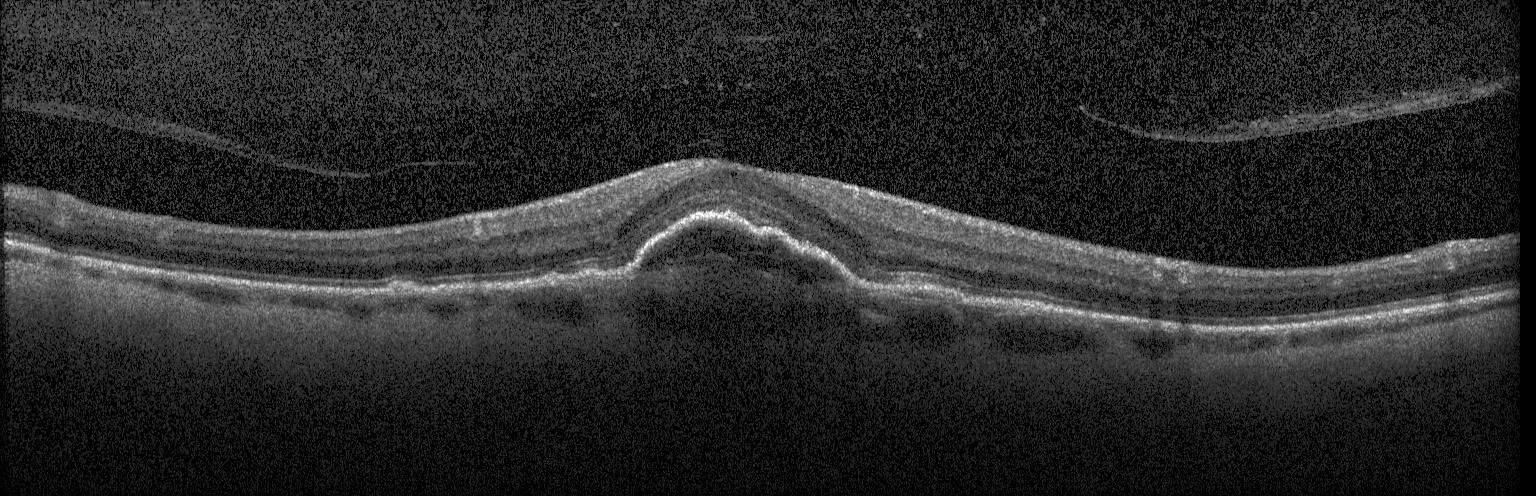 Diagnosis: a choroidal neovascular membrane.